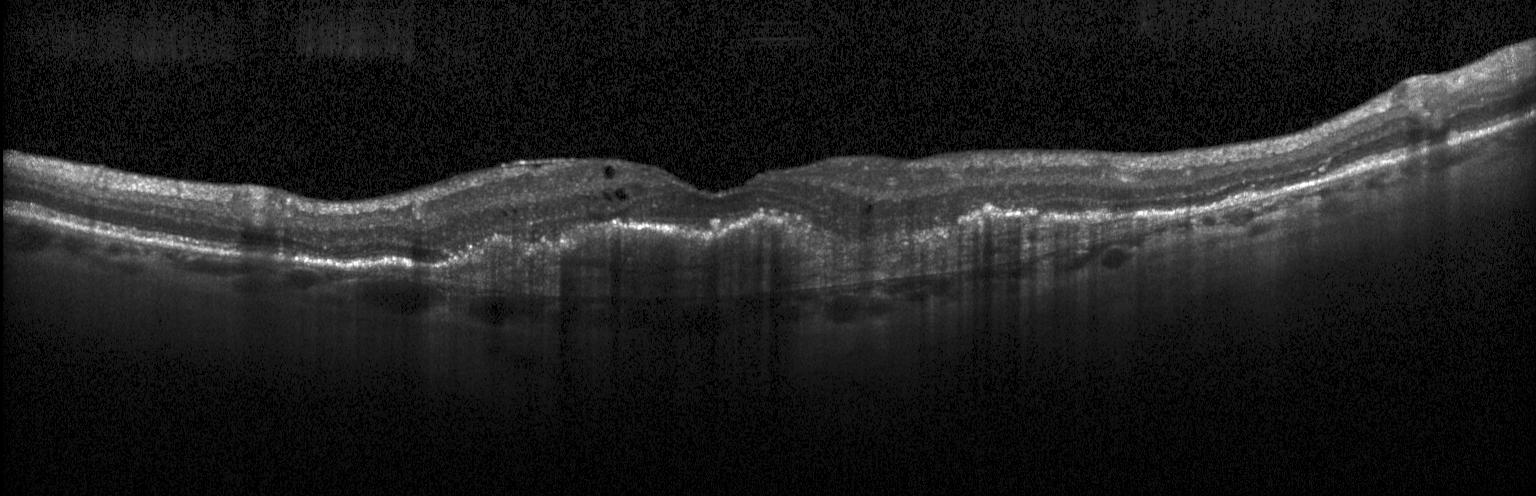

Assessment: a choroidal neovascular membrane.